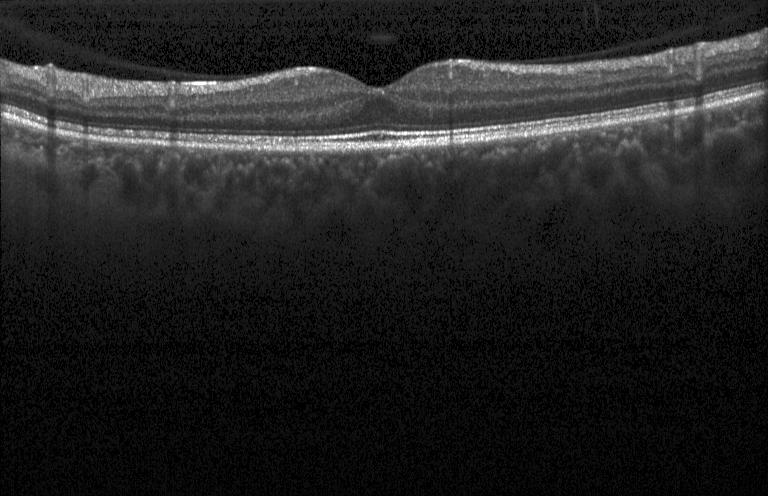

Retinal OCT cross-section; spectral-domain OCT — The scan shows no choroidal neovascularization, no diabetic macular edema, and no drusen.